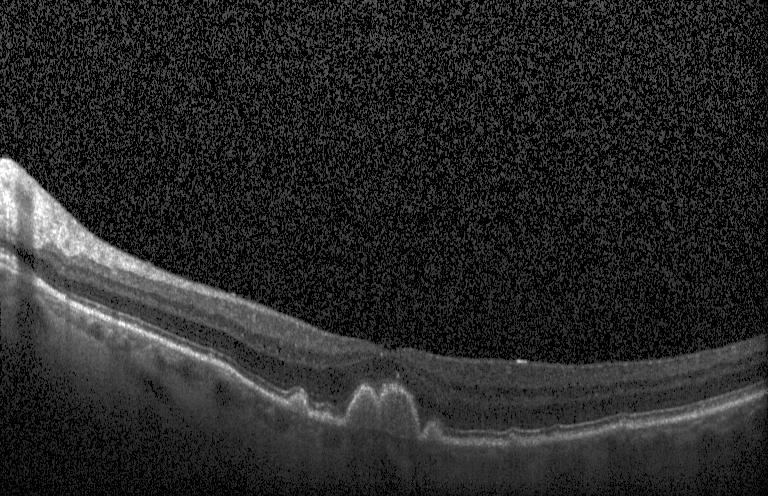
Diagnosis: sub-RPE drusenoid deposits.